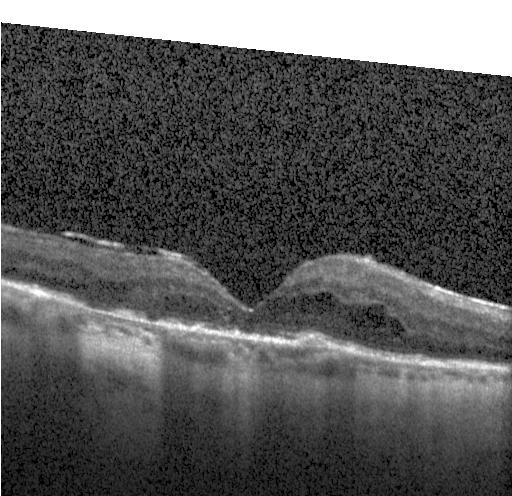

Heidelberg Spectralis; retinal OCT B-scan; spectral-domain OCT; through the macula
Diagnosis: diabetic macular edema (DME).